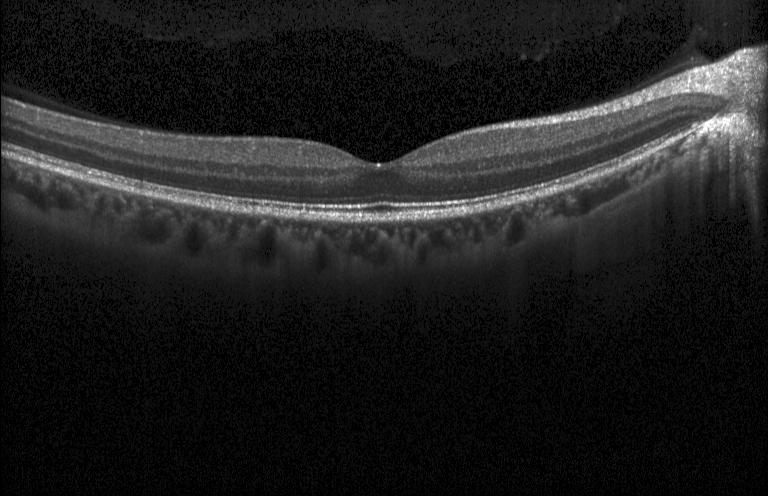
The scan shows no CNV, no DME, and no drusen.